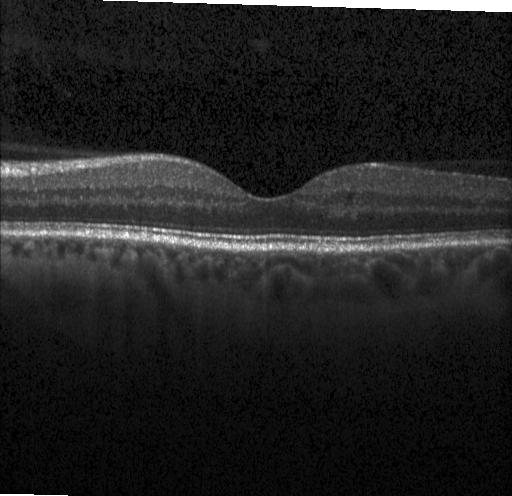

Retinal OCT cross-section. Dx: no choroidal neovascularization, diabetic macular edema, or drusen.